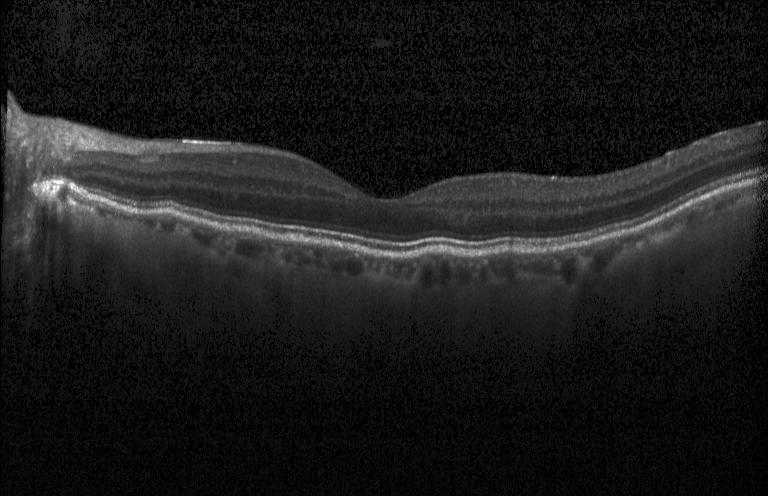

OCT B-scan
Impression: no choroidal neovascularization, no diabetic macular edema, and no drusen.